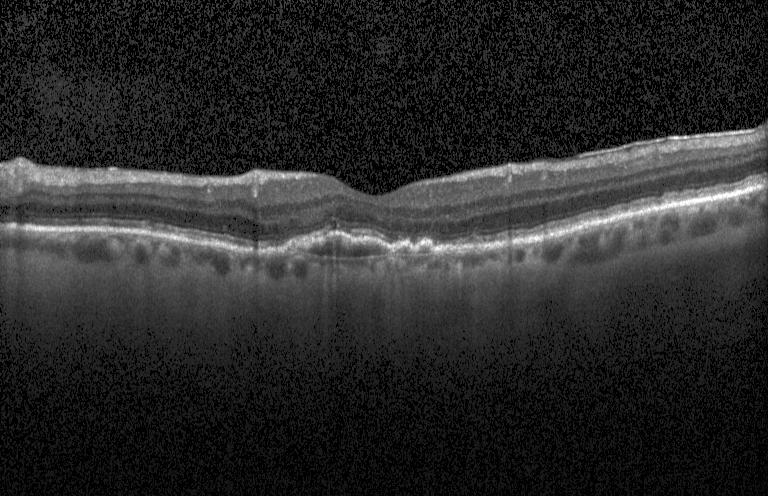

Retinal OCT cross-section · SD-OCT · centered on the fovea. Dx: CNV.